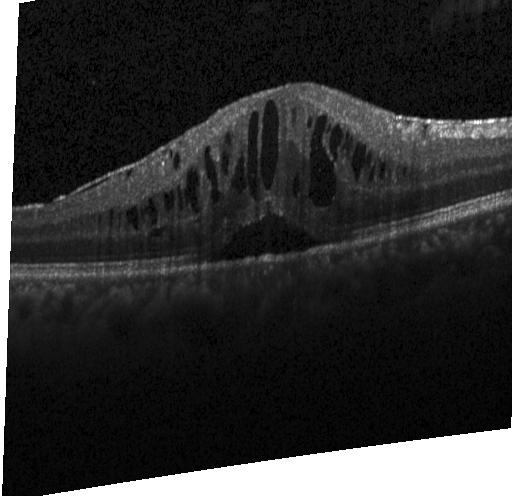 Spectral-domain optical coherence tomography · retinal OCT B-scan. Impression: diabetic macular edema.